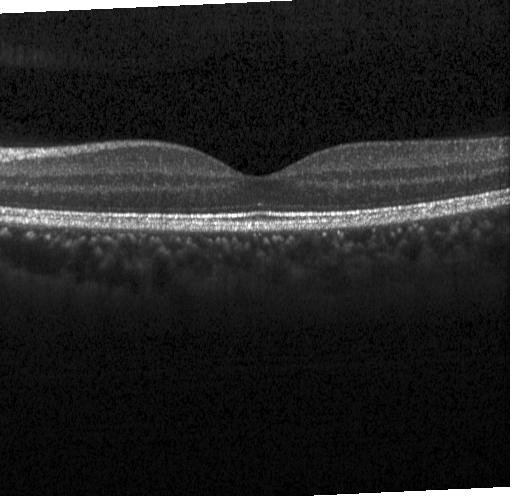

OCT B-scan
The scan shows no evidence of choroidal neovascularization, diabetic macular edema, or drusen.